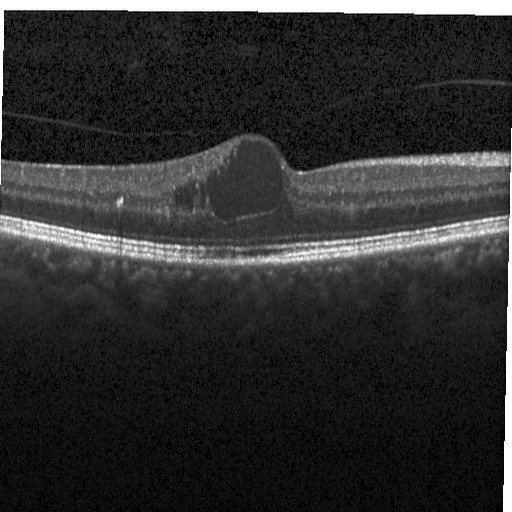 Macular OCT: diabetic macular edema.